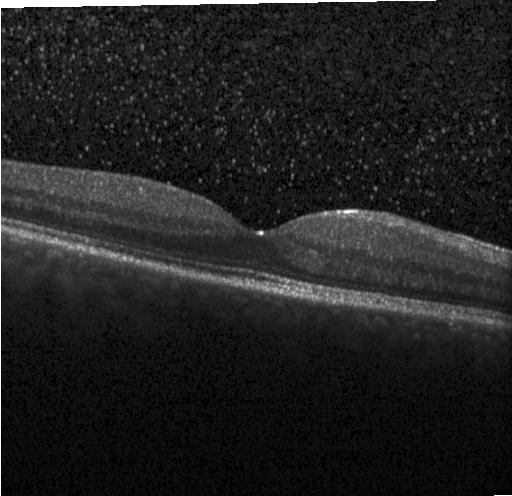

Diagnosis: no evidence of CNV, DME, or drusen.